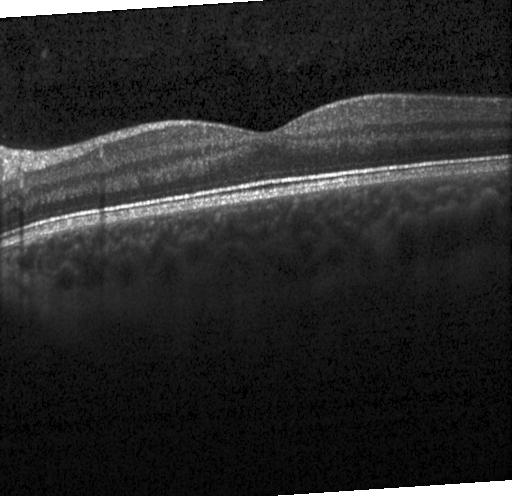

Retinal OCT B-scan. Impression: neither CNV, DME, nor drusen.